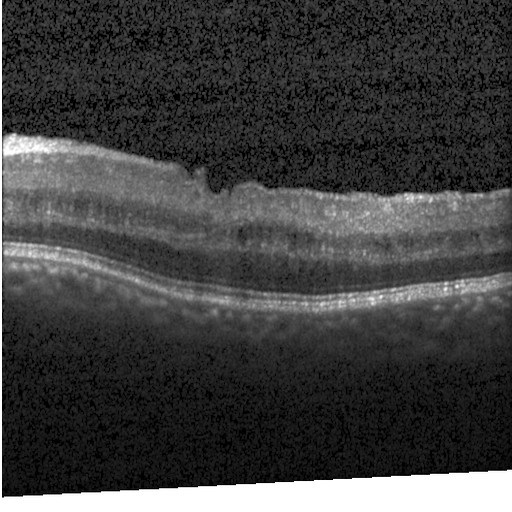 Optical coherence tomography scan
Finding: diabetic macular edema.